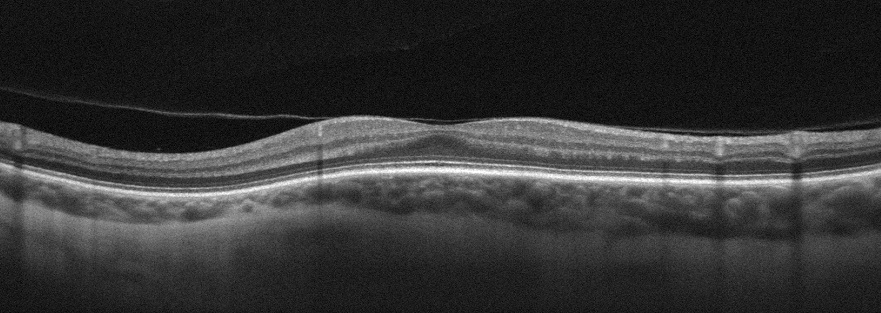
Optovue Avanti RTVue XR. Optical coherence tomography scan. Impression: no evidence of AMD, DME, ERM, RAO, RVO, or VID.